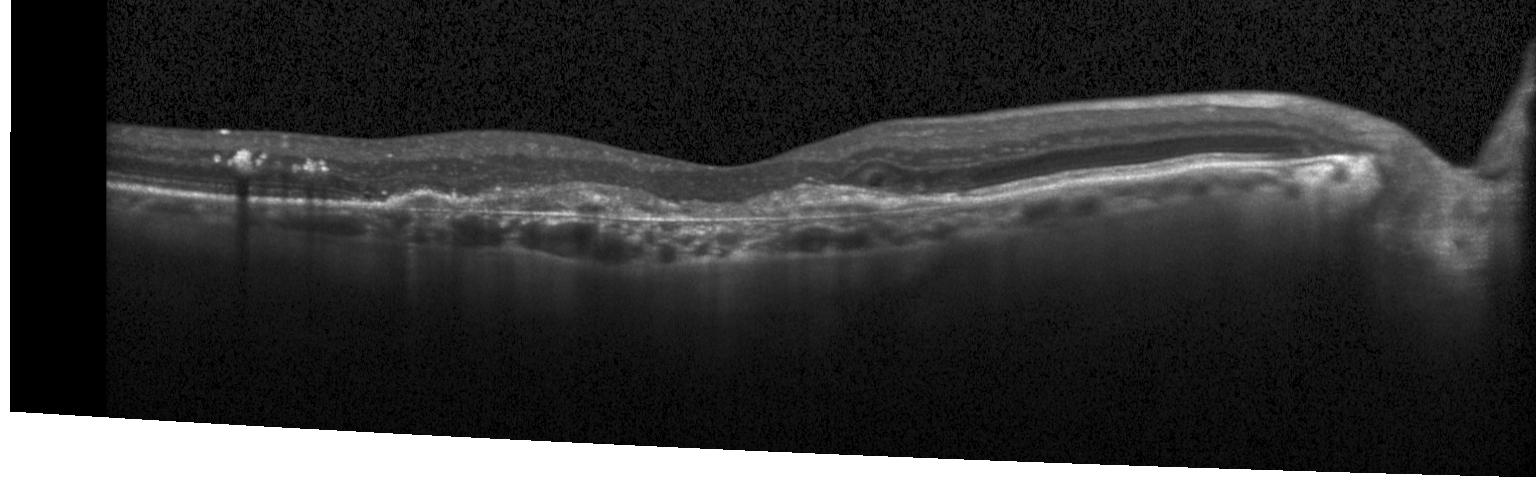
Optical coherence tomography scan — Dx: a choroidal neovascular membrane.